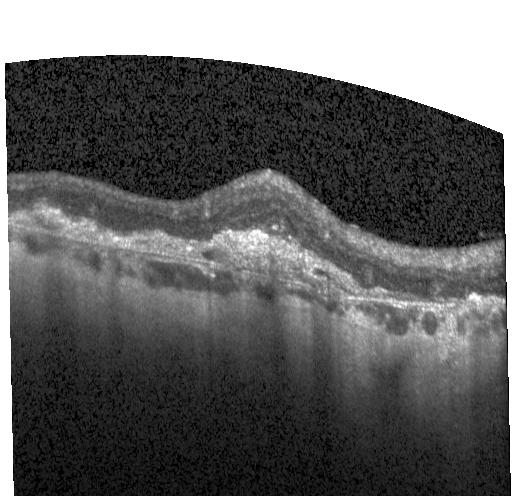
Spectral-domain OCT, retinal OCT B-scan, fovea-centered, instrument: Heidelberg Spectralis
OCT finding: choroidal neovascularization.